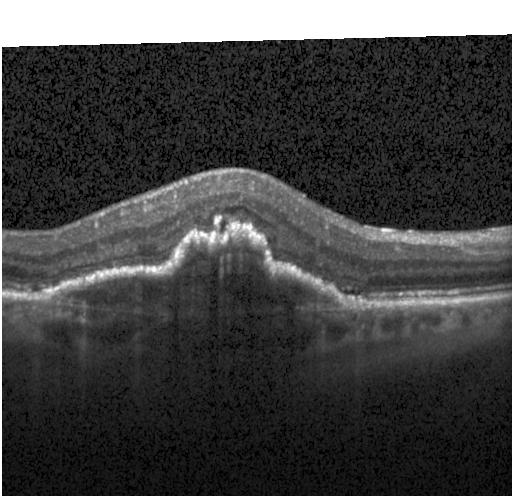

Impression: a choroidal neovascular membrane.